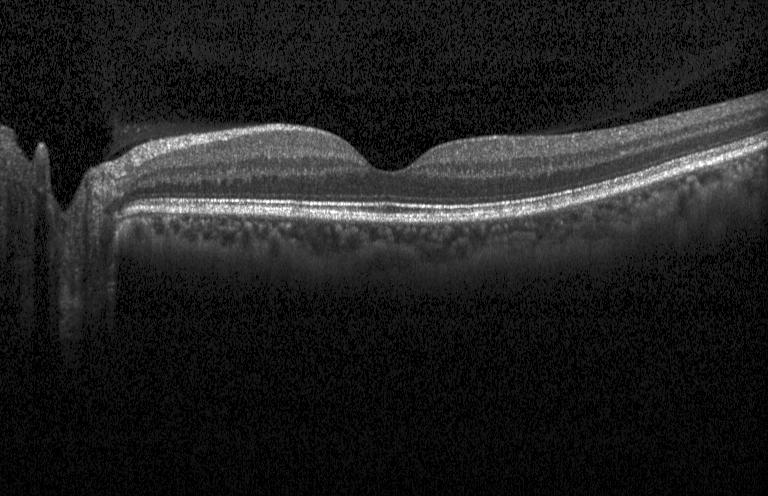
Fovea-centered · OCT B-scan · spectral-domain OCT
Assessment: no choroidal neovascularization, diabetic macular edema, or drusen.